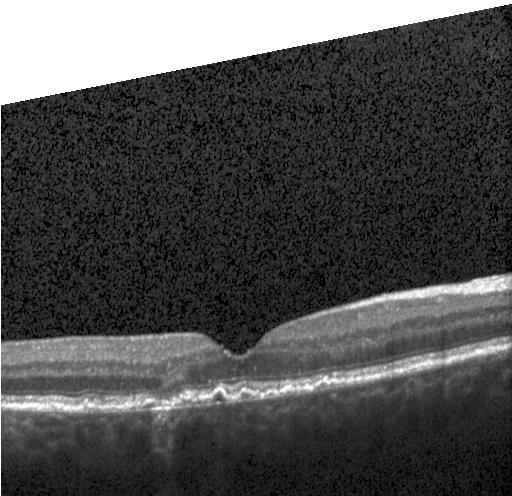

Optical coherence tomography B-scan; centered on the fovea; SD-OCT; Heidelberg Spectralis OCT system — Impression: a choroidal neovascular membrane.